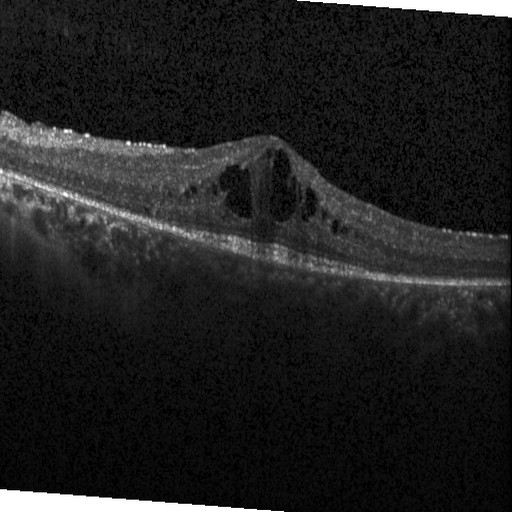 Spectral-domain OCT B-scan: diabetic macular edema (DME).